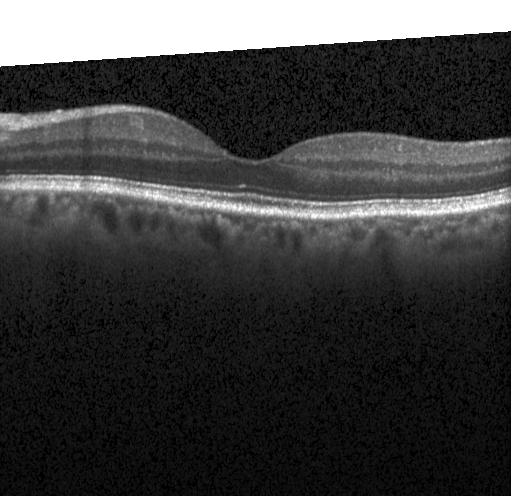

Diagnosis: no evidence of choroidal neovascularization, diabetic macular edema, or drusen.